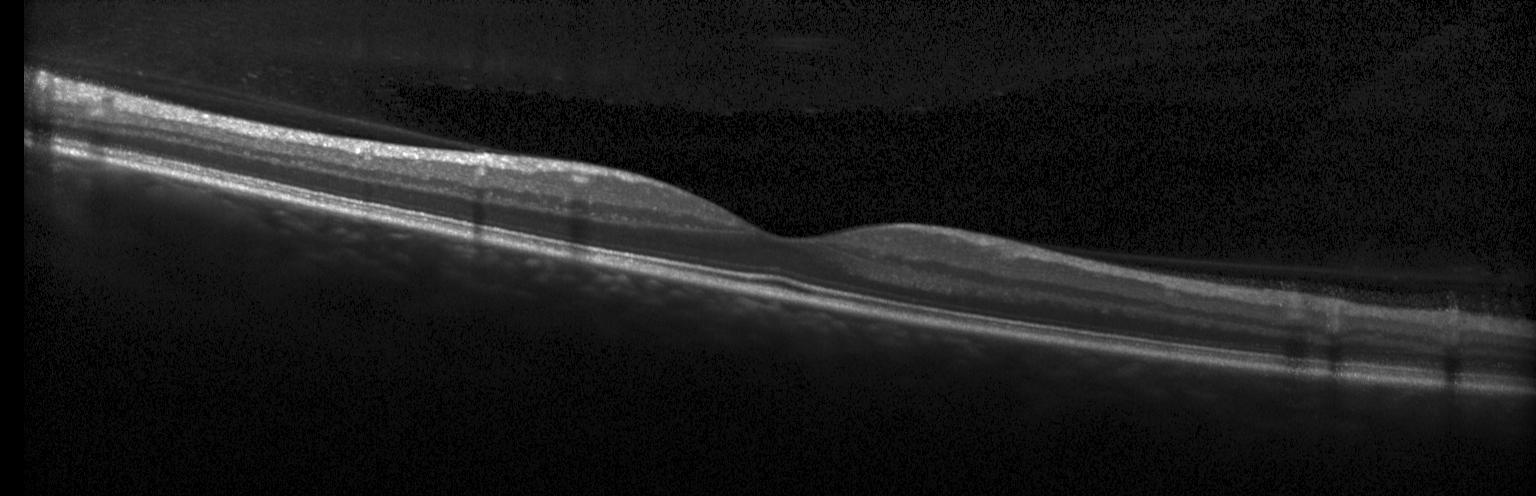
Retinal OCT cross-section
The scan shows no evidence of choroidal neovascularization, diabetic macular edema, or drusen.